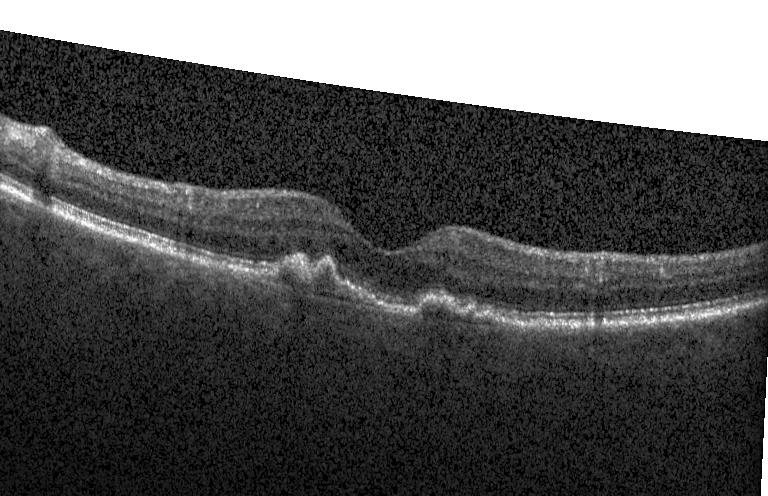

Retinal OCT cross-section, fovea-centered, instrument: Heidelberg Spectralis.
A choroidal neovascular membrane.